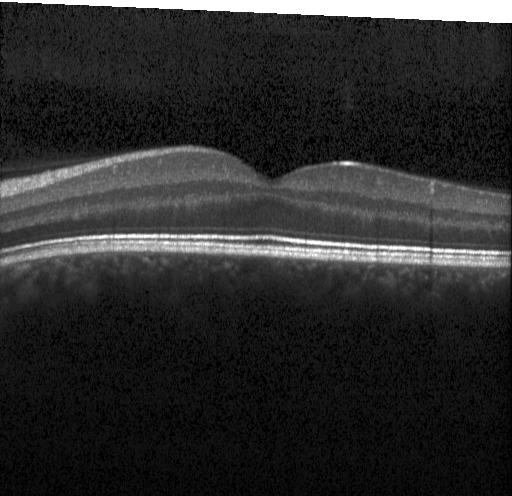
Impression: no choroidal neovascularization, diabetic macular edema, or drusen.